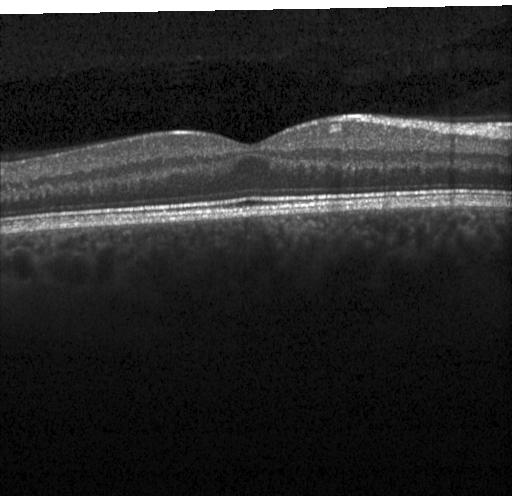 Optical coherence tomography B-scan. Diagnosis: no choroidal neovascularization, diabetic macular edema, or drusen.